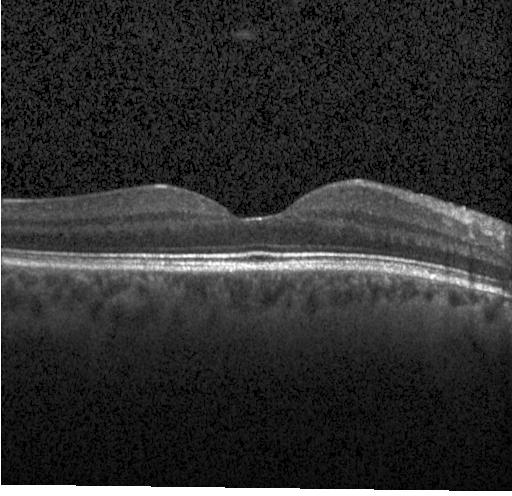
OCT scan showing no evidence of choroidal neovascularization, diabetic macular edema, or drusen.